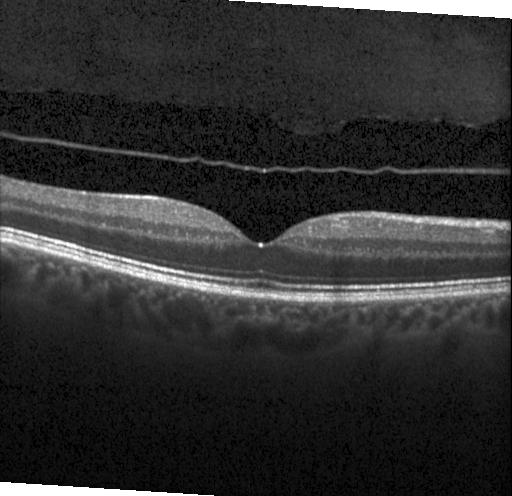 Diagnosis: no choroidal neovascularization, diabetic macular edema, or drusen.